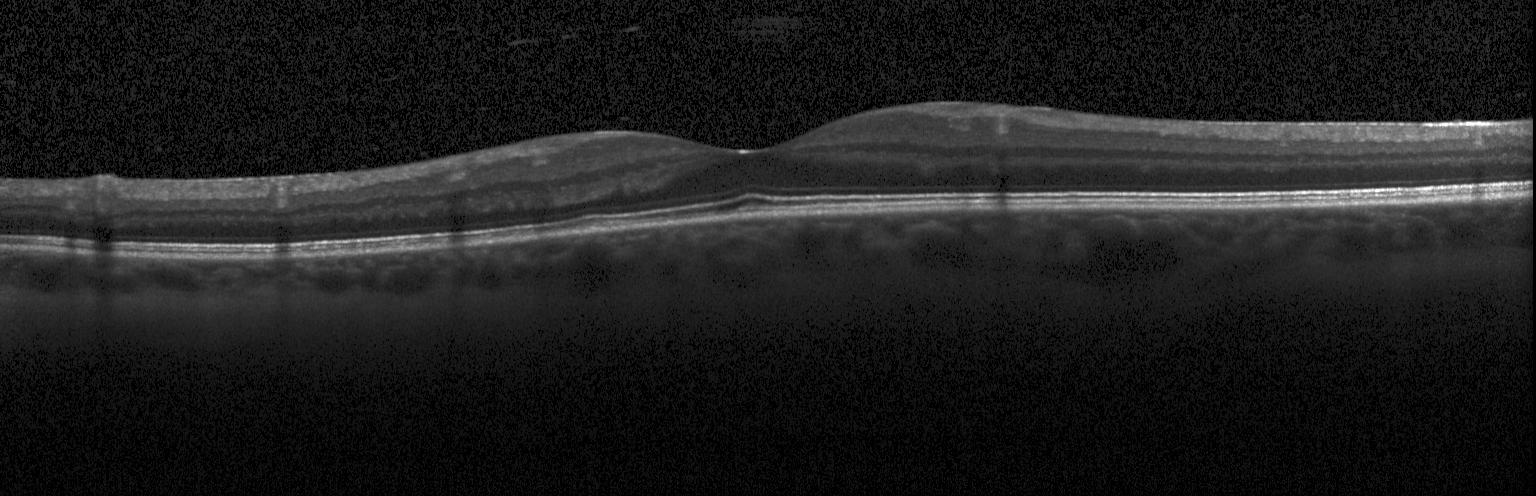

Retinal OCT B-scan
Macular OCT: no evidence of CNV, DME, or drusen.